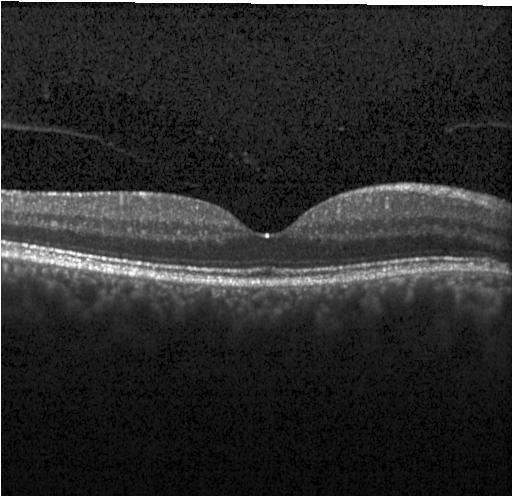
Optical coherence tomography B-scan; SD-OCT. Dx: neither choroidal neovascularization, diabetic macular edema, nor drusen.